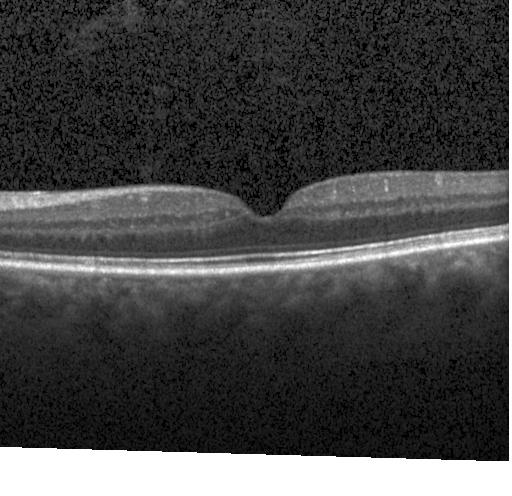 Instrument: Heidelberg Spectralis. OCT B-scan. Spectral-domain OCT.
Dx: no choroidal neovascularization, diabetic macular edema, or drusen.